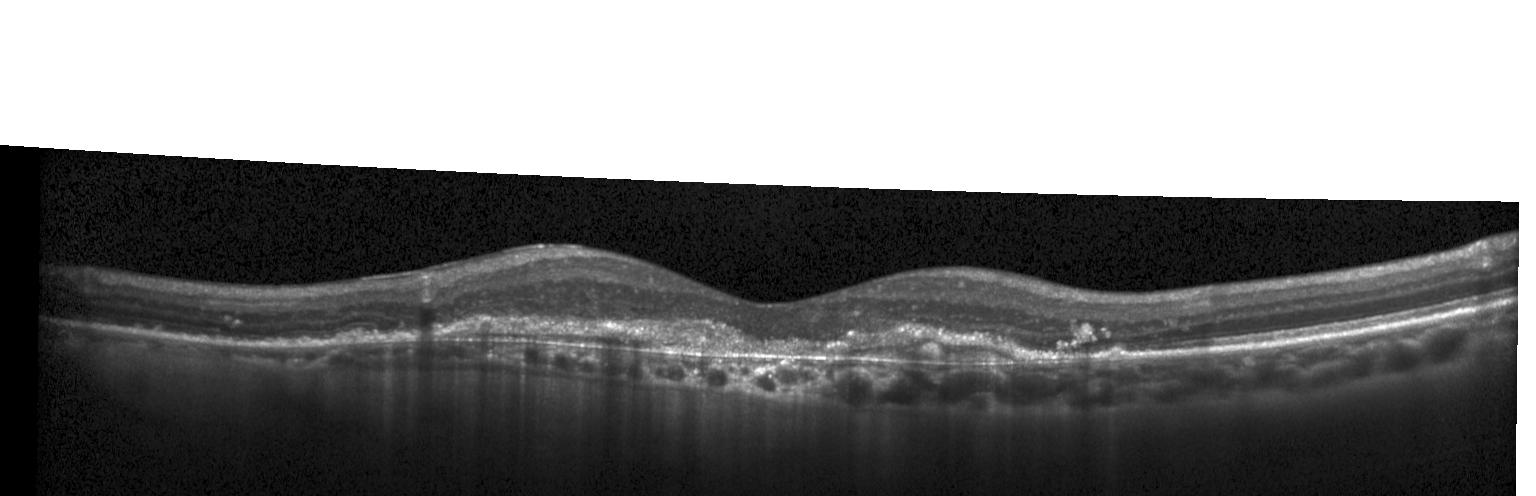

Spectral-domain OCT B-scan: choroidal neovascularization (CNV).